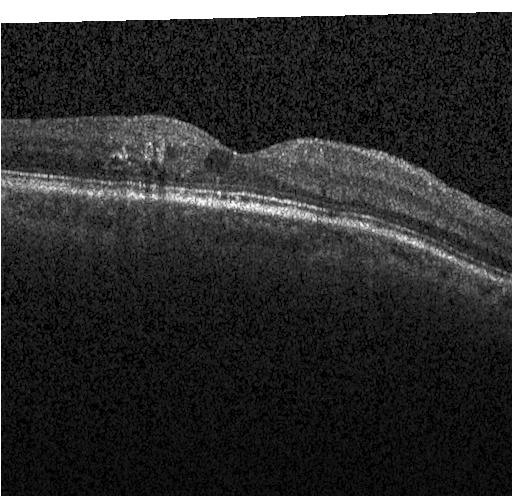 OCT finding: diabetic macular edema (DME).